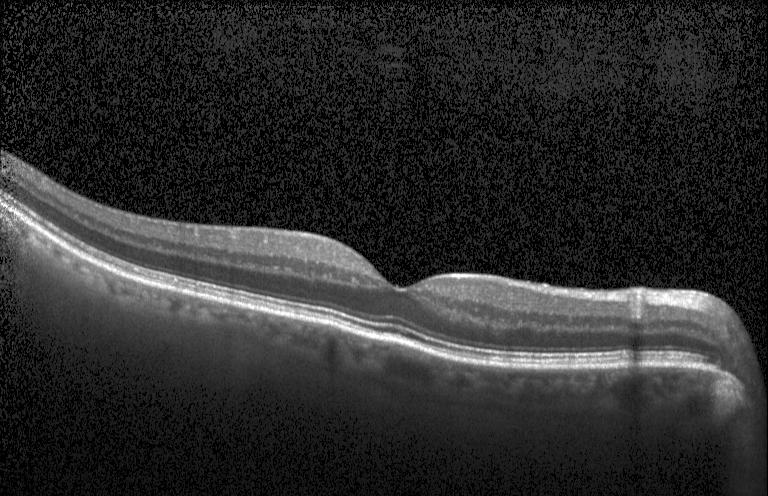

Acquired on a Heidelberg Spectralis · SD-OCT · horizontal scan through the fovea · retinal OCT B-scan — The scan shows no evidence of CNV, DME, or drusen.